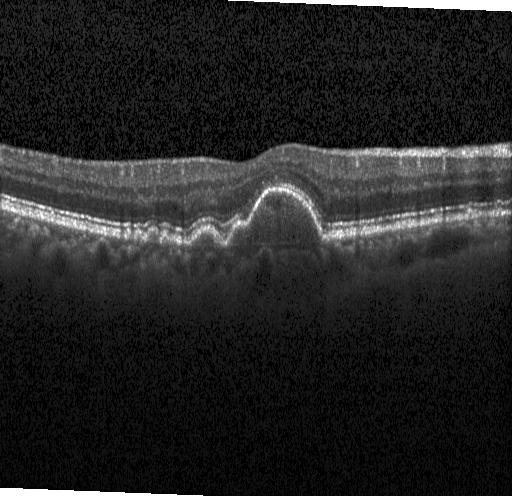
Fovea-centered; instrument: Heidelberg Spectralis; spectral-domain optical coherence tomography; optical coherence tomography scan — Dx: sub-RPE drusenoid deposits.